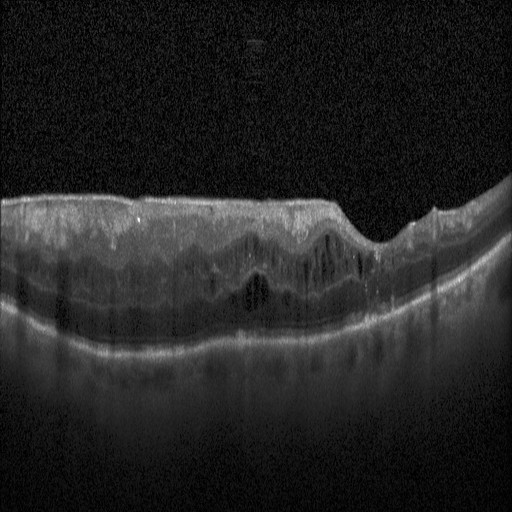

Spectral-domain optical coherence tomography, OCT line scan, Heidelberg Spectralis OCT system, centered on the fovea — Macular OCT: diabetic macular edema (DME).